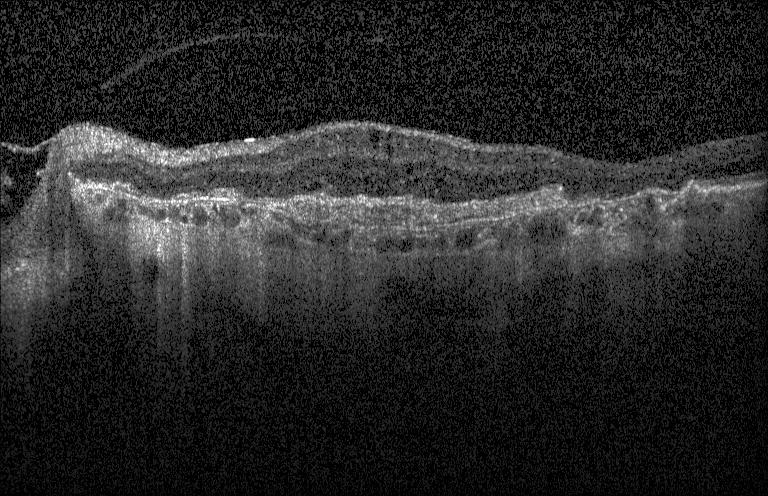 Retinal OCT cross-section. Spectral-domain OCT. The scan shows choroidal neovascularization.